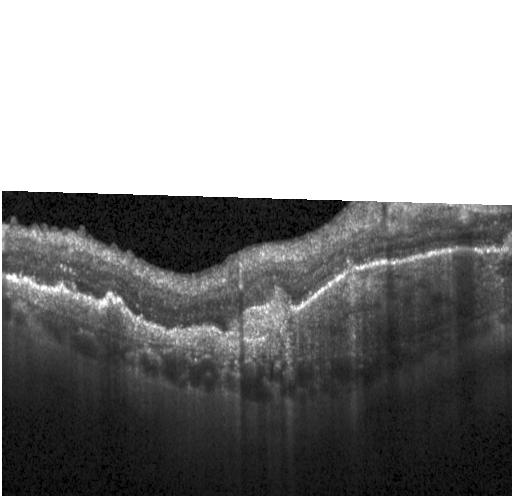
Centered on the fovea · retinal OCT B-scan · Heidelberg Spectralis
Diagnosis: CNV.